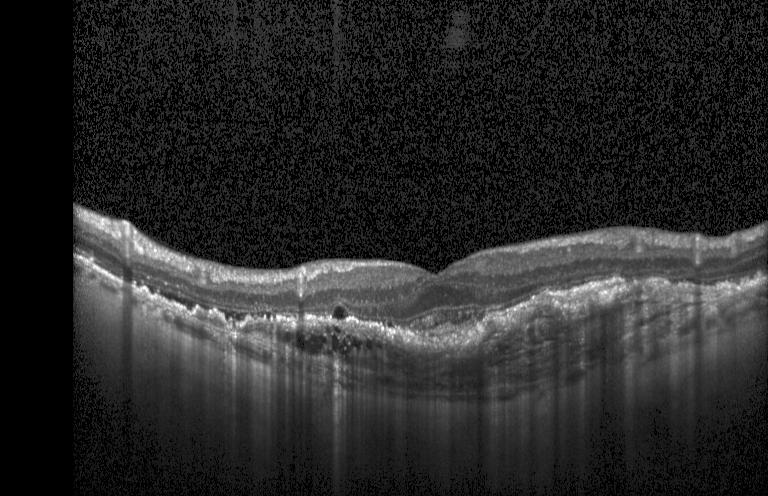
Retinal OCT cross-section showing a choroidal neovascular membrane.